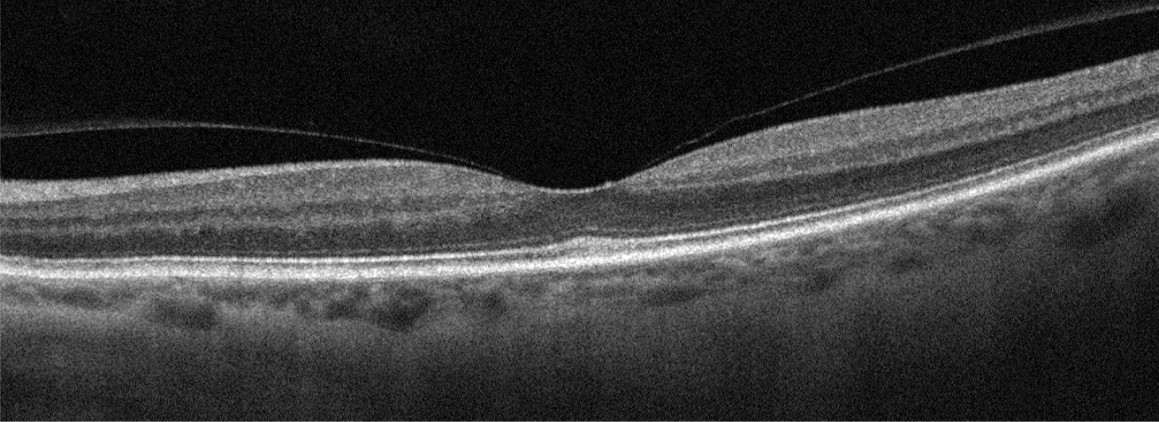
OCT B-scan showing no AMD, DME, ERM, RAO, RVO, or VID.